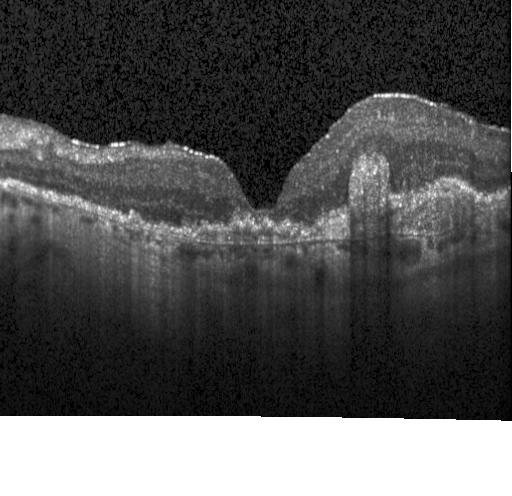

Impression: choroidal neovascularization (CNV).